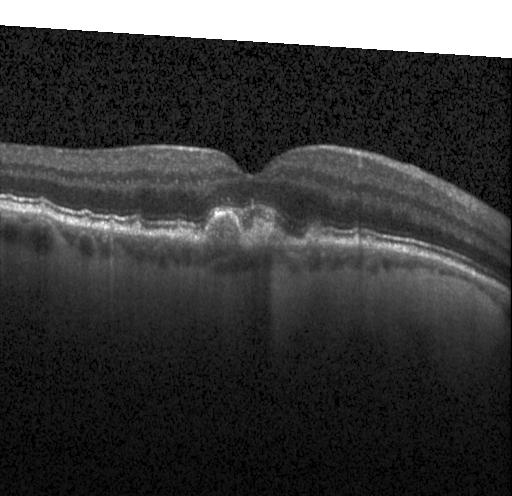

Dx: sub-RPE drusenoid deposits.